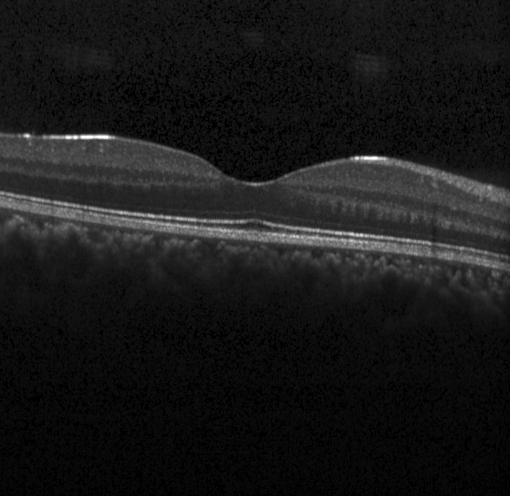
Optical coherence tomography scan. Macular OCT: no evidence of choroidal neovascularization, diabetic macular edema, or drusen.